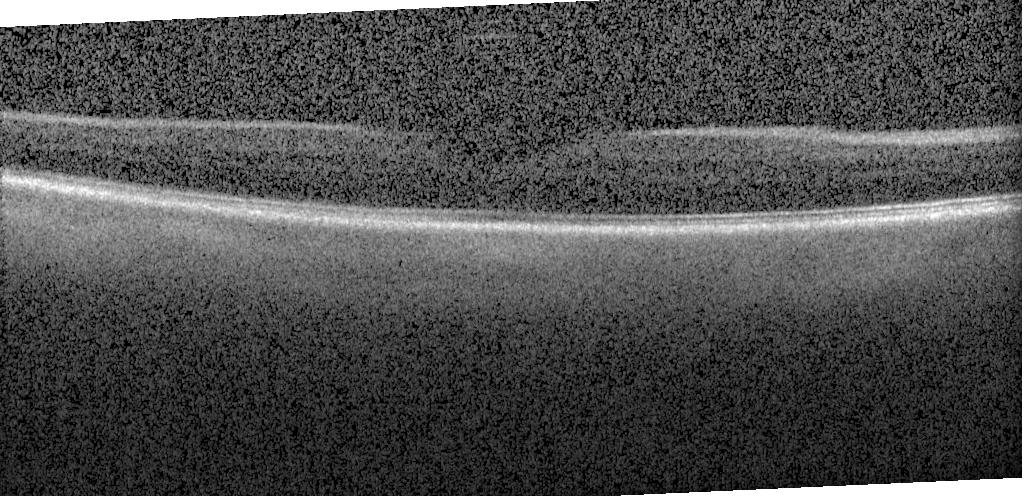
SD-OCT, horizontal scan through the fovea, OCT B-scan.
Diagnosis: no CNV, no DME, and no drusen.